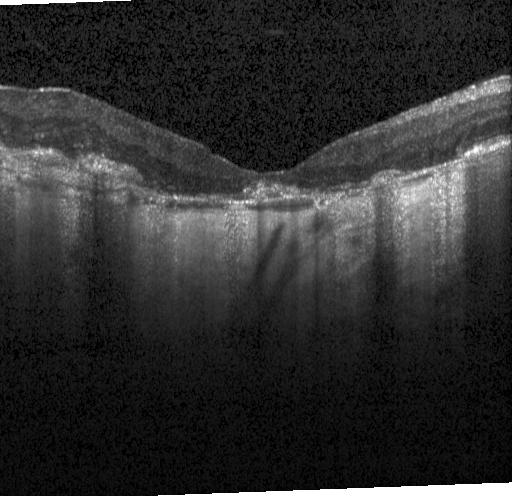

OCT B-scan showing CNV.